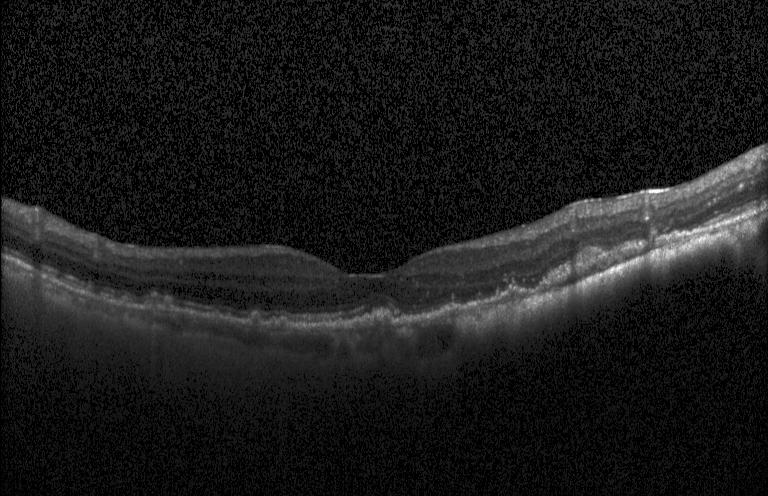 Spectral-domain OCT B-scan: choroidal neovascularization (CNV).